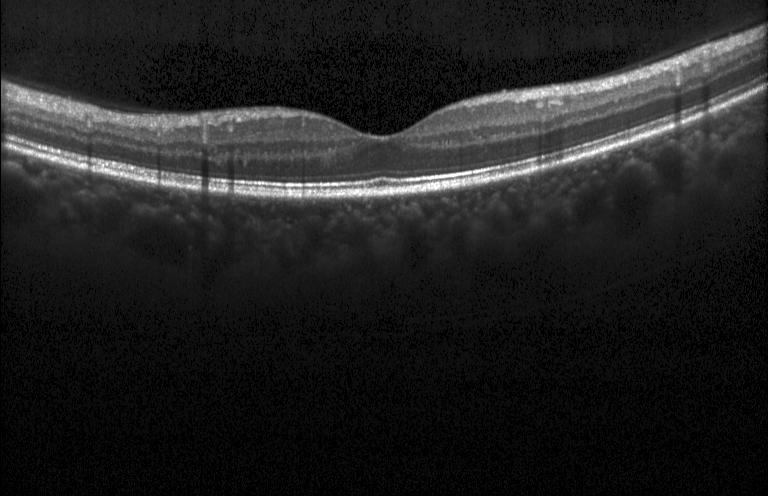 Macular OCT: neither choroidal neovascularization, diabetic macular edema, nor drusen.